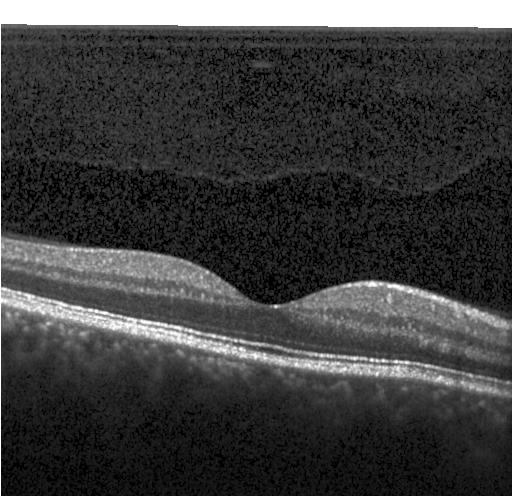 Finding: no choroidal neovascularization, no diabetic macular edema, and no drusen.